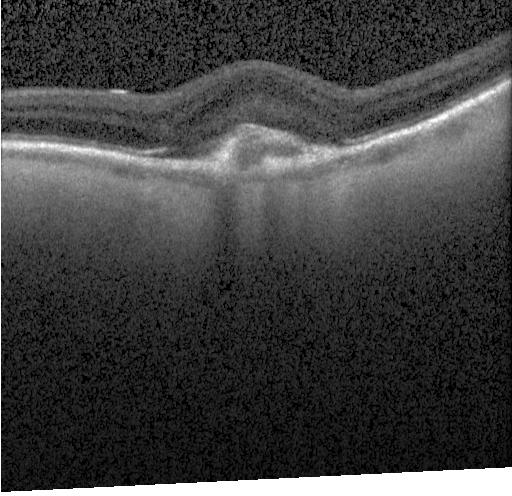 OCT B-scan. A choroidal neovascular membrane.